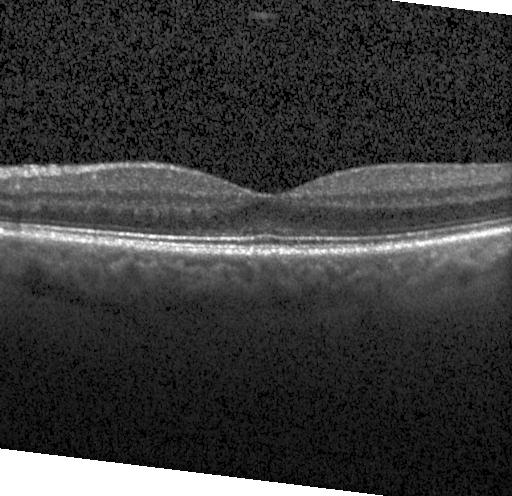
Diagnosis: no choroidal neovascularization, diabetic macular edema, or drusen.